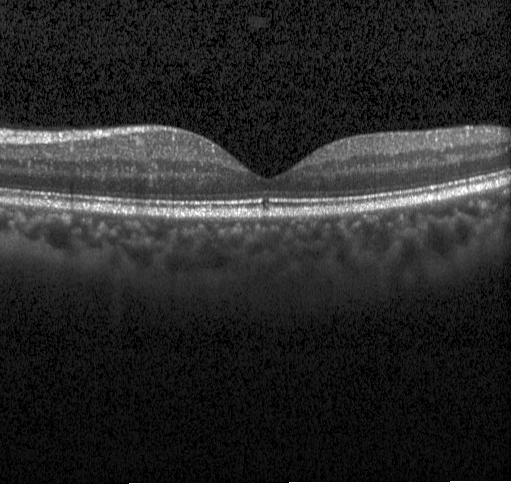
OCT finding: no evidence of choroidal neovascularization, diabetic macular edema, or drusen.